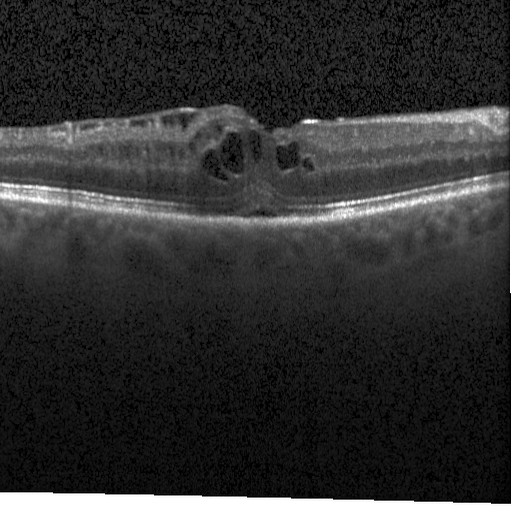

Diagnosis: diabetic macular edema (DME).